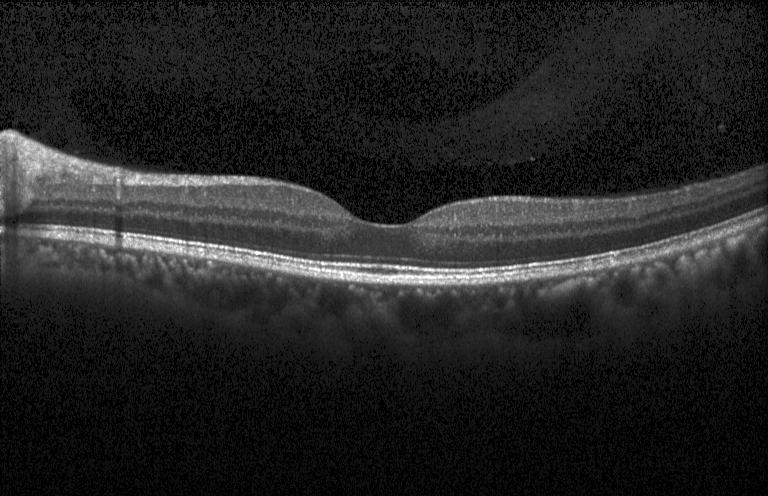

Macular OCT: no CNV, DME, or drusen.